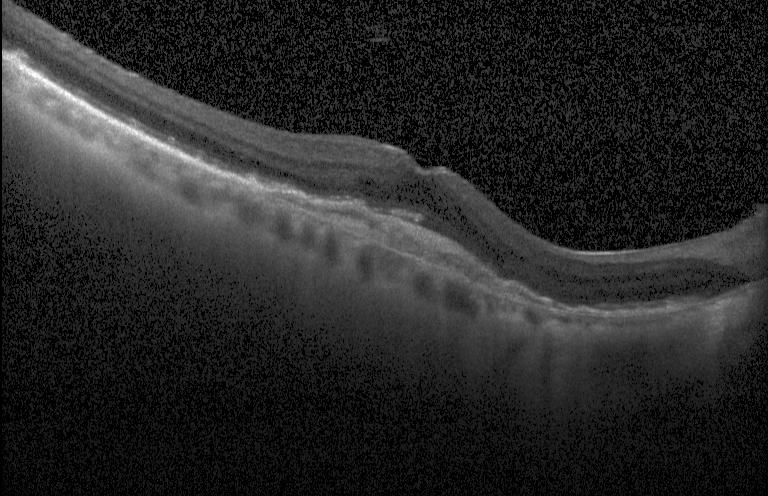
Optical coherence tomography scan · Heidelberg Spectralis · fovea-centered
This B-scan demonstrates a choroidal neovascular membrane.